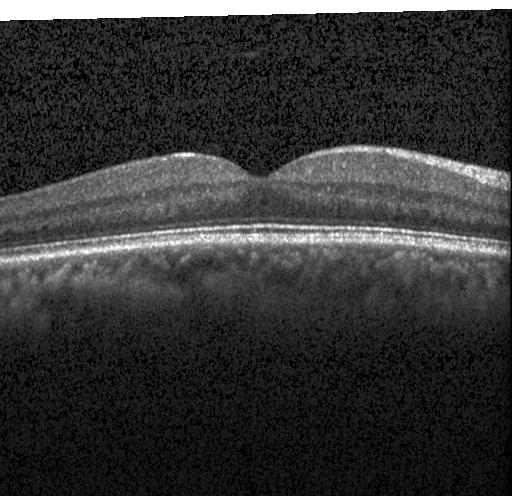
Spectral-domain OCT; OCT B-scan; horizontal scan through the fovea; Heidelberg Spectralis OCT system — OCT finding: no choroidal neovascularization, no diabetic macular edema, and no drusen.